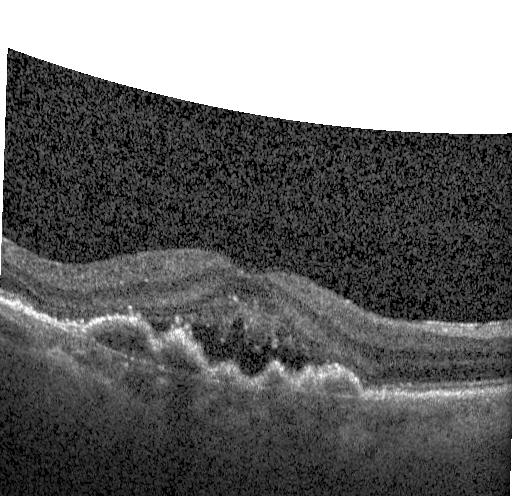 Instrument: Heidelberg Spectralis, OCT B-scan.
Diagnosis: choroidal neovascularization.